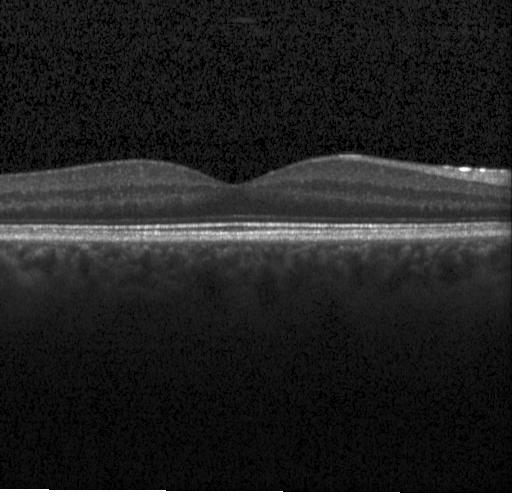

OCT line scan. Spectral-domain OCT. Heidelberg Spectralis OCT system. Horizontal scan through the fovea
OCT finding: no evidence of CNV, DME, or drusen.